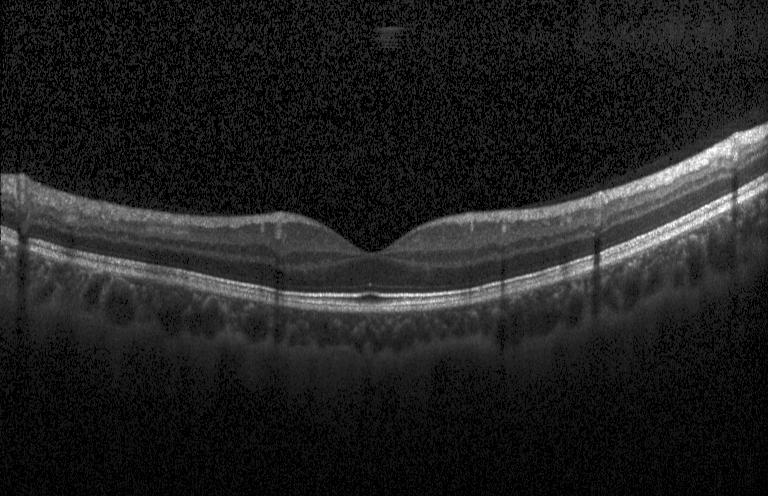 Diagnosis: no CNV, DME, or drusen.